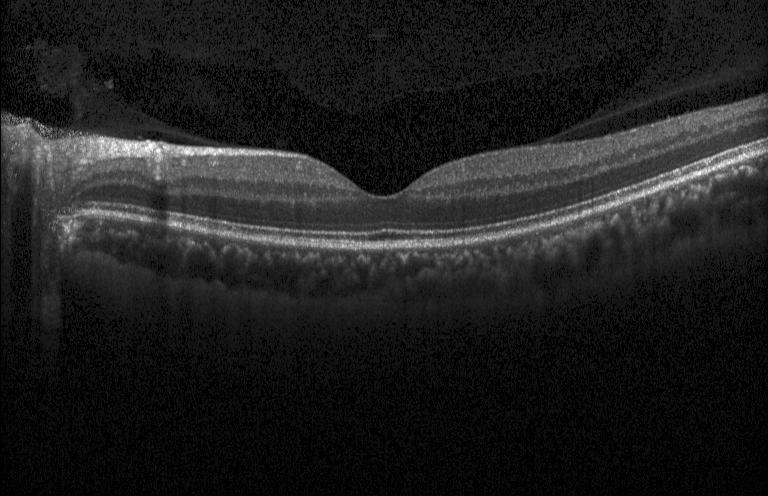
Impression: no evidence of choroidal neovascularization, diabetic macular edema, or drusen.